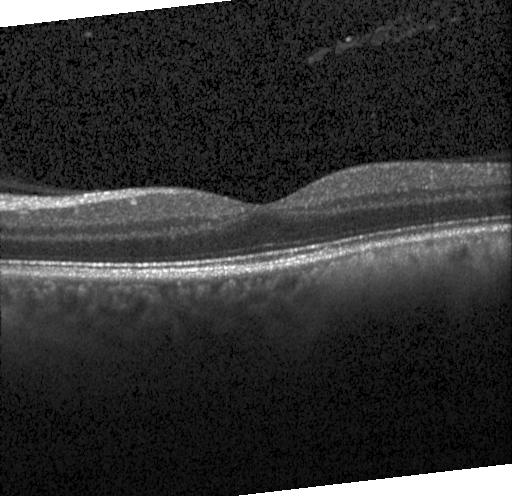

Finding: no choroidal neovascularization, no diabetic macular edema, and no drusen.